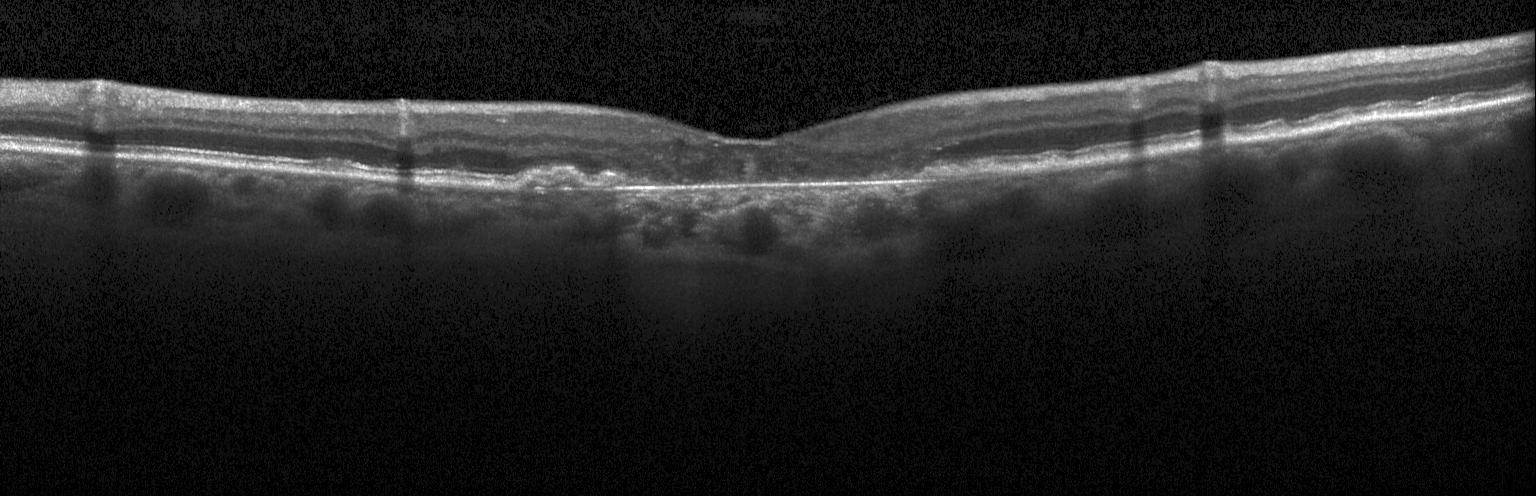 Finding: choroidal neovascularization.